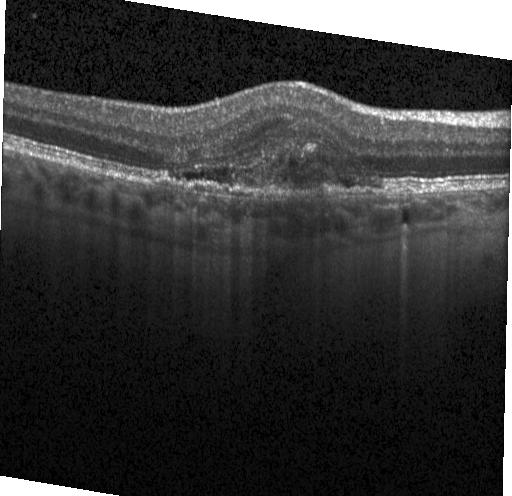
Assessment: a choroidal neovascular membrane.